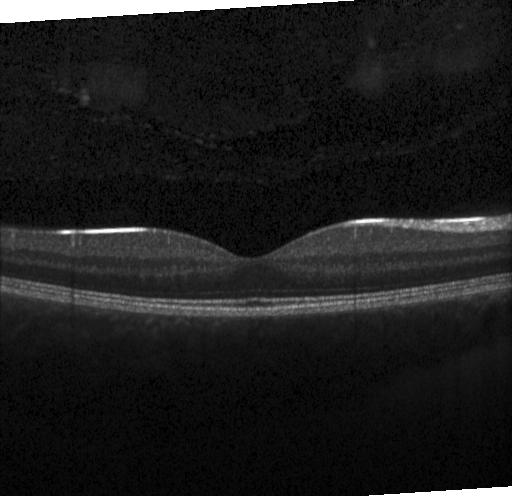
Retinal OCT B-scan, SD-OCT, acquired on a Heidelberg Spectralis, fovea-centered. No choroidal neovascularization, no diabetic macular edema, and no drusen.